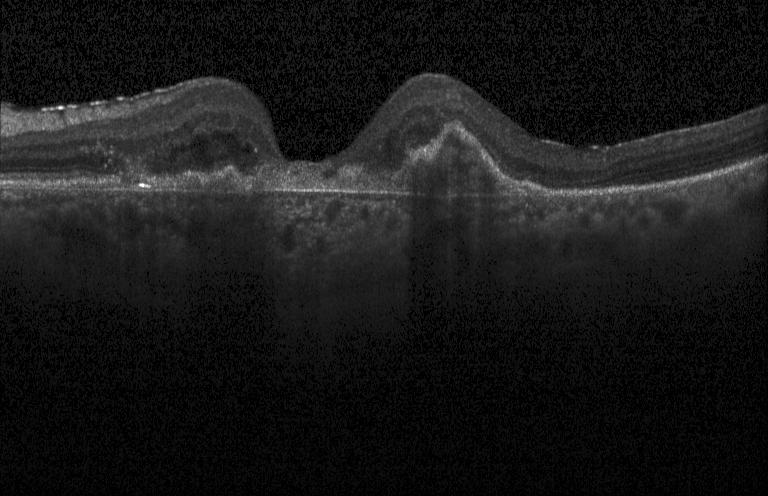 Impression: a choroidal neovascular membrane.